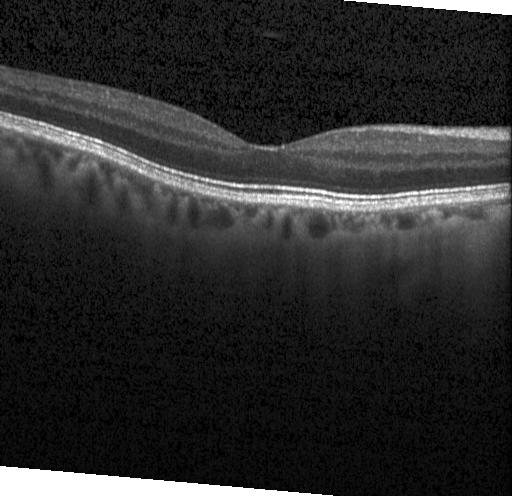
Horizontal scan through the fovea. Retinal OCT B-scan — Finding: no choroidal neovascularization, no diabetic macular edema, and no drusen.